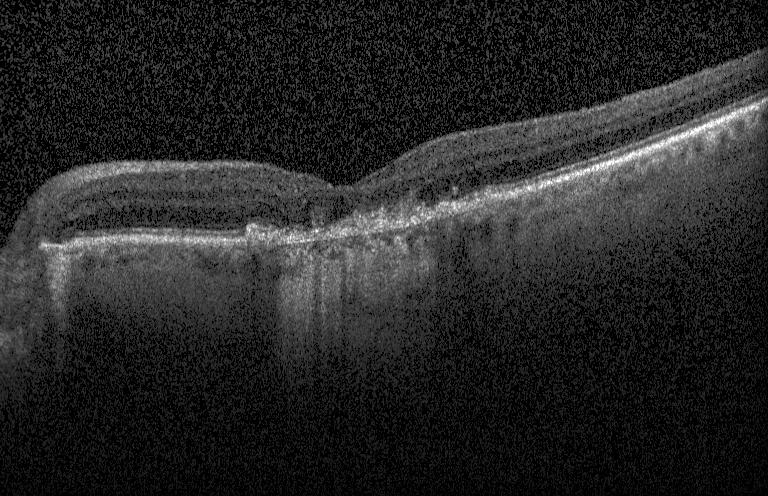

Diagnosis: a choroidal neovascular membrane.